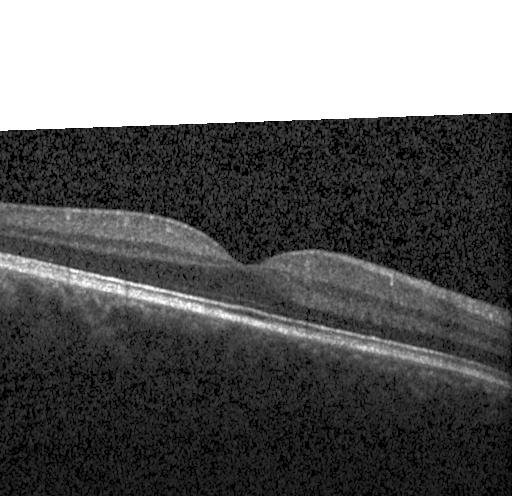

Dx: no evidence of CNV, DME, or drusen.